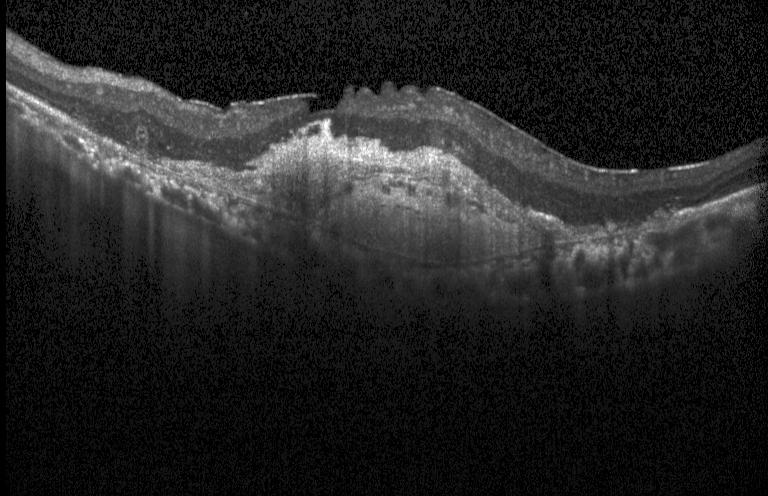
Macular OCT demonstrating CNV.